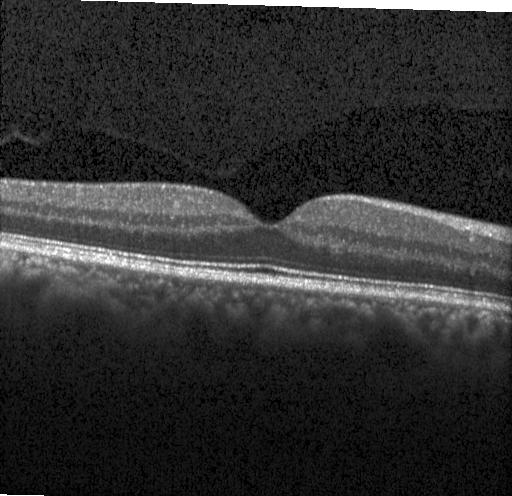

Centered on the fovea, spectral-domain OCT, optical coherence tomography B-scan — Diagnosis: no choroidal neovascularization, diabetic macular edema, or drusen.